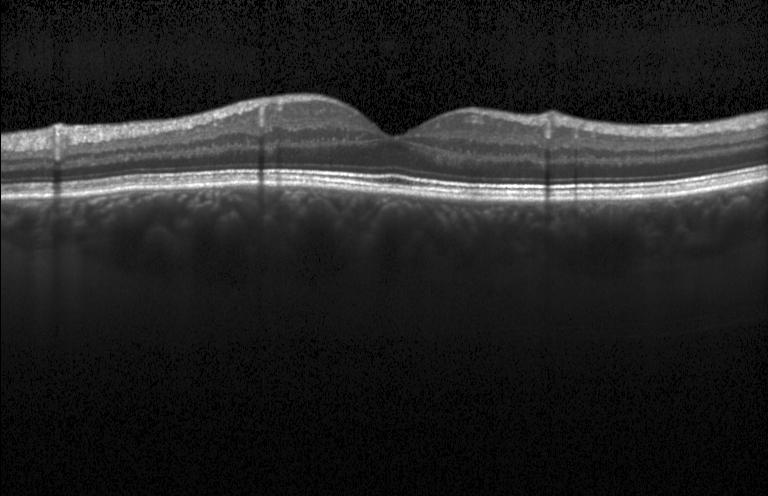
Macular scan, optical coherence tomography B-scan.
Diagnosis: no evidence of CNV, DME, or drusen.